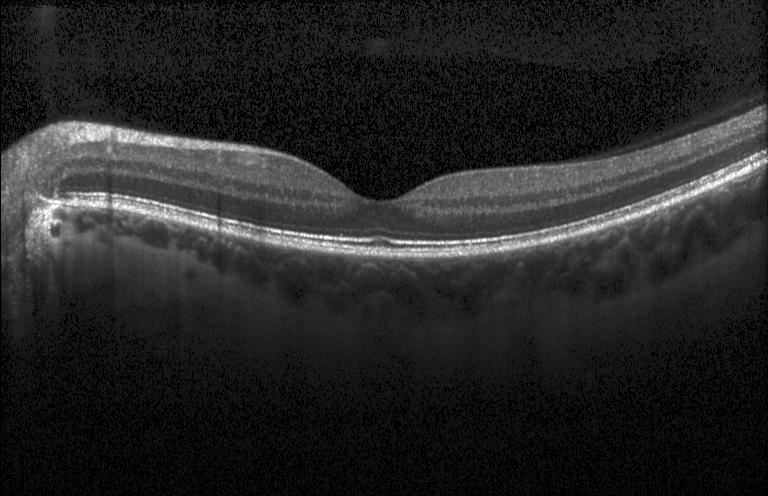
OCT scan showing no choroidal neovascularization, no diabetic macular edema, and no drusen.